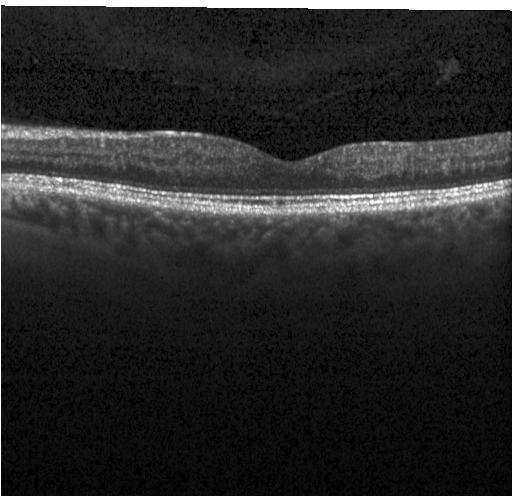

Optical coherence tomography B-scan · SD-OCT.
Diagnosis: no evidence of CNV, DME, or drusen.